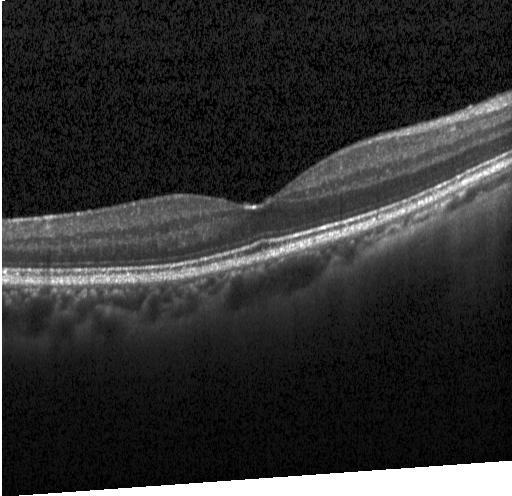

Retinal OCT cross-section · fovea-centered · acquired on a Heidelberg Spectralis · spectral-domain optical coherence tomography.
Macular OCT: no evidence of CNV, DME, or drusen.